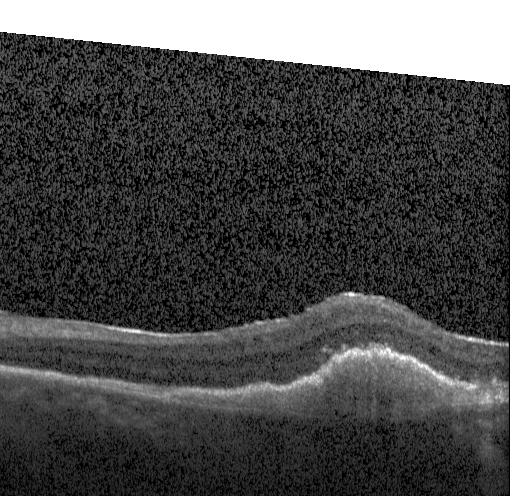
Impression: a choroidal neovascular membrane.